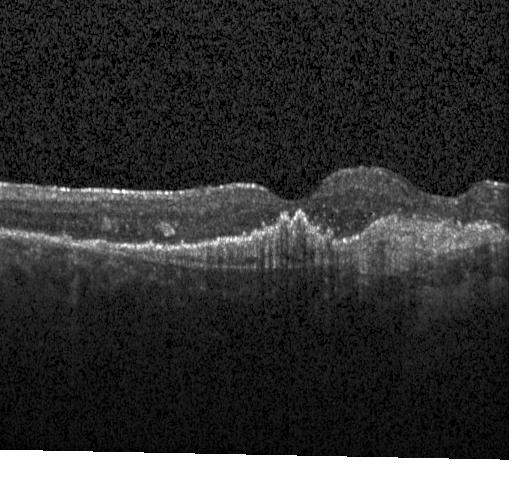
Diagnosis: a choroidal neovascular membrane.